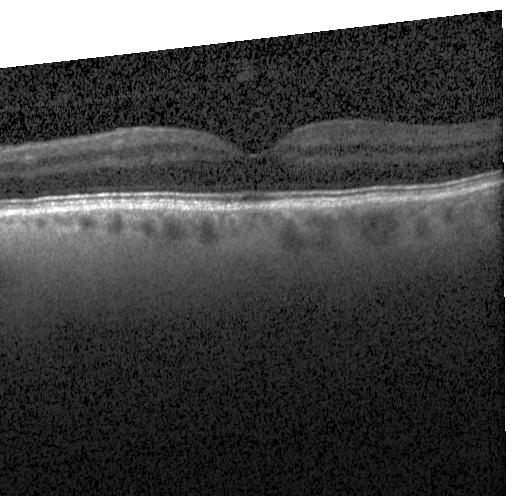 The scan shows no choroidal neovascularization, no diabetic macular edema, and no drusen.